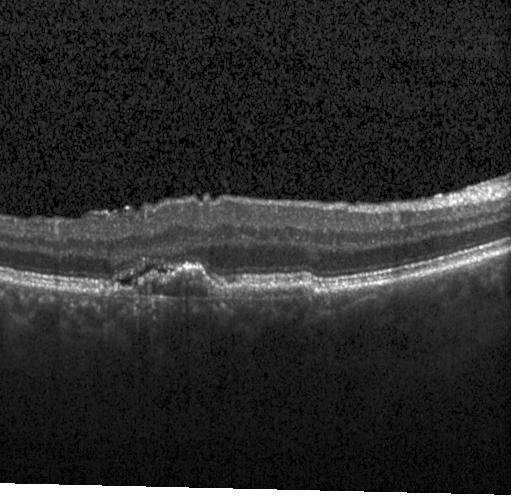
Optical coherence tomography B-scan. Instrument: Heidelberg Spectralis. Spectral-domain OCT. Finding: a choroidal neovascular membrane.